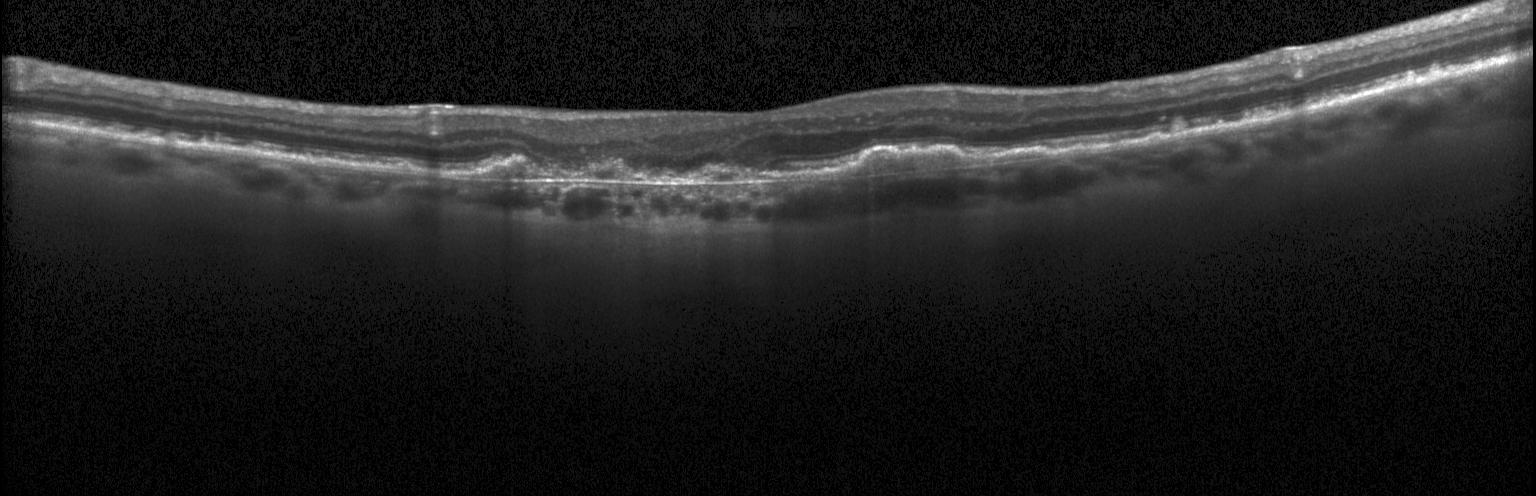

Finding: a choroidal neovascular membrane.